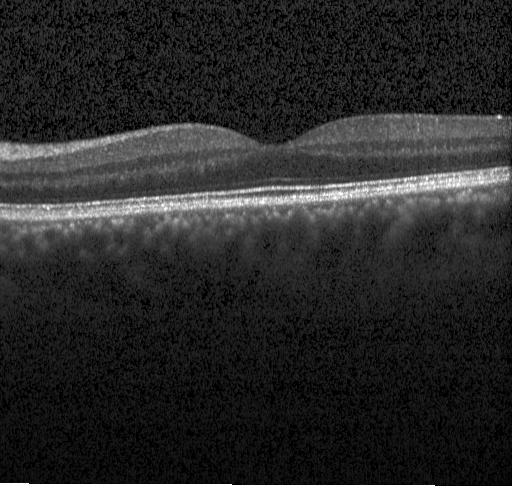 Fovea-centered; OCT line scan — The scan shows no choroidal neovascularization, no diabetic macular edema, and no drusen.